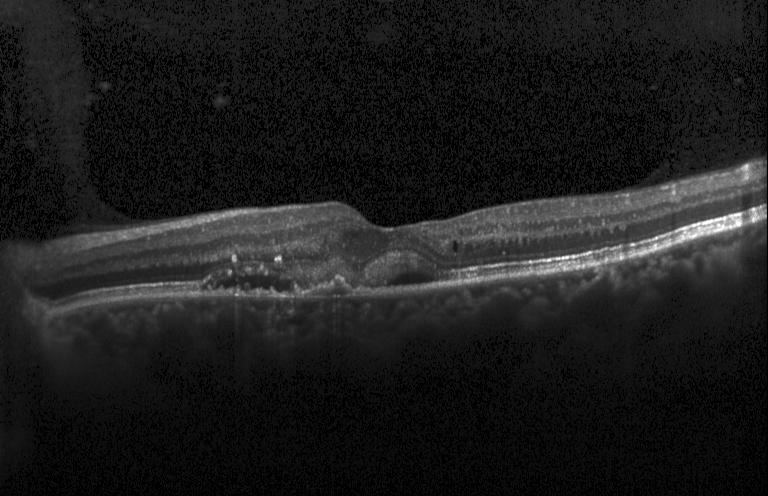
Optical coherence tomography B-scan; through the macula
Finding: choroidal neovascularization.